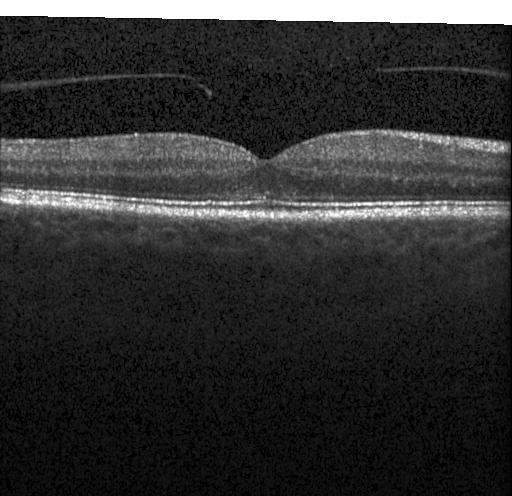 Diagnosis: no choroidal neovascularization, no diabetic macular edema, and no drusen.